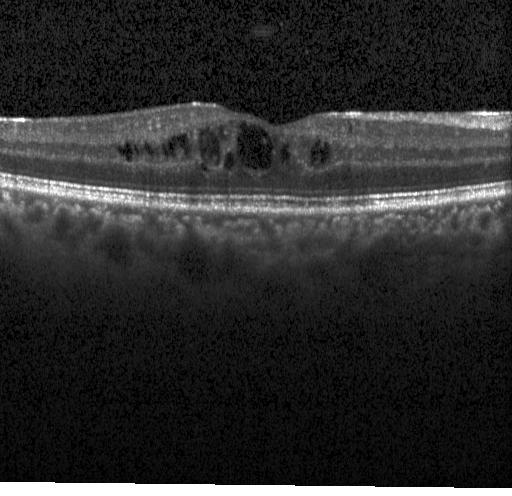
Optical coherence tomography scan. Spectral-domain optical coherence tomography — Impression: DME.